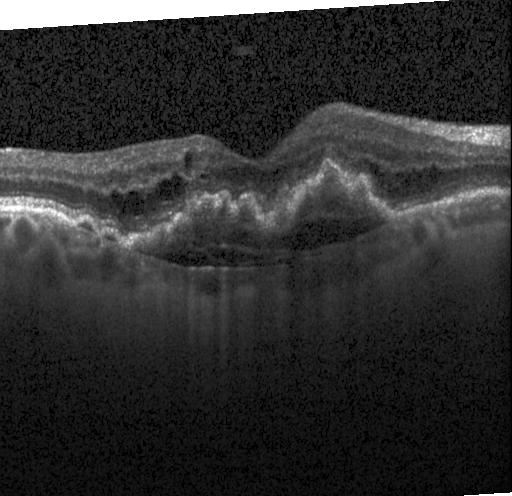
Impression: choroidal neovascularization.